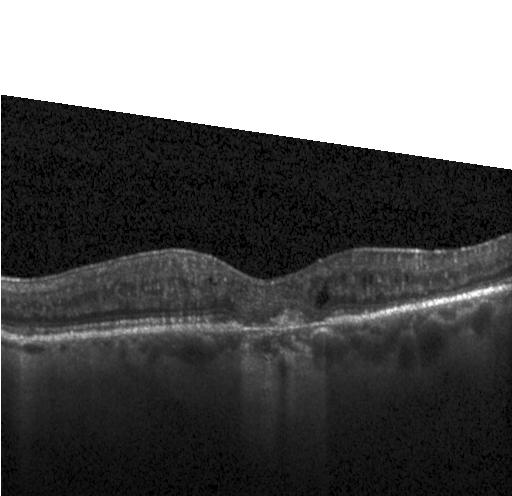
OCT B-scan · spectral-domain OCT · instrument: Heidelberg Spectralis · macular scan — Macular OCT: choroidal neovascularization (CNV).